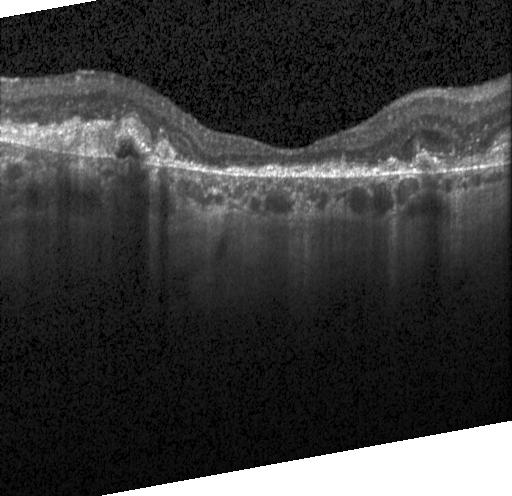 Spectral-domain optical coherence tomography · acquired on a Heidelberg Spectralis · through the macula · OCT line scan
Macular OCT: choroidal neovascularization (CNV).